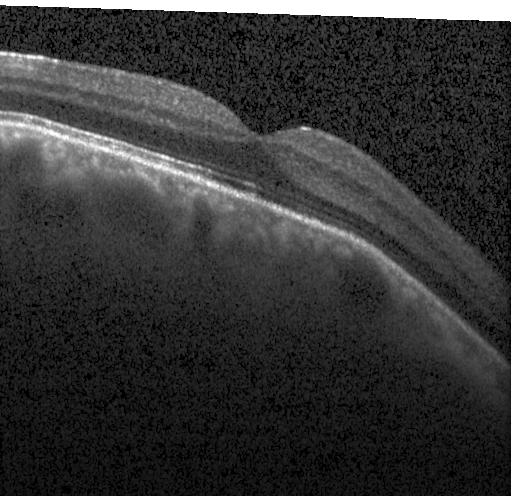

Spectral-domain optical coherence tomography · through the macula · OCT line scan · Heidelberg Spectralis OCT system — This B-scan demonstrates no choroidal neovascularization, diabetic macular edema, or drusen.